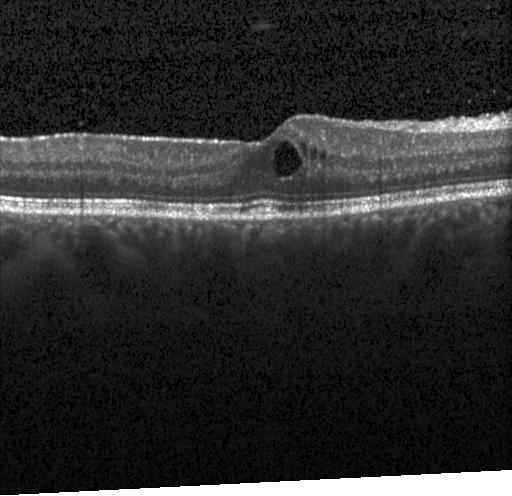 OCT B-scan — Diagnosis: DME.